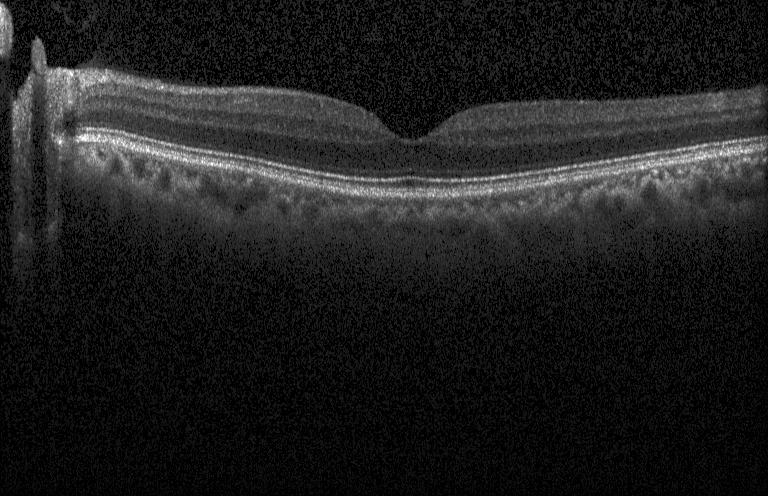

This B-scan demonstrates no evidence of choroidal neovascularization, diabetic macular edema, or drusen.